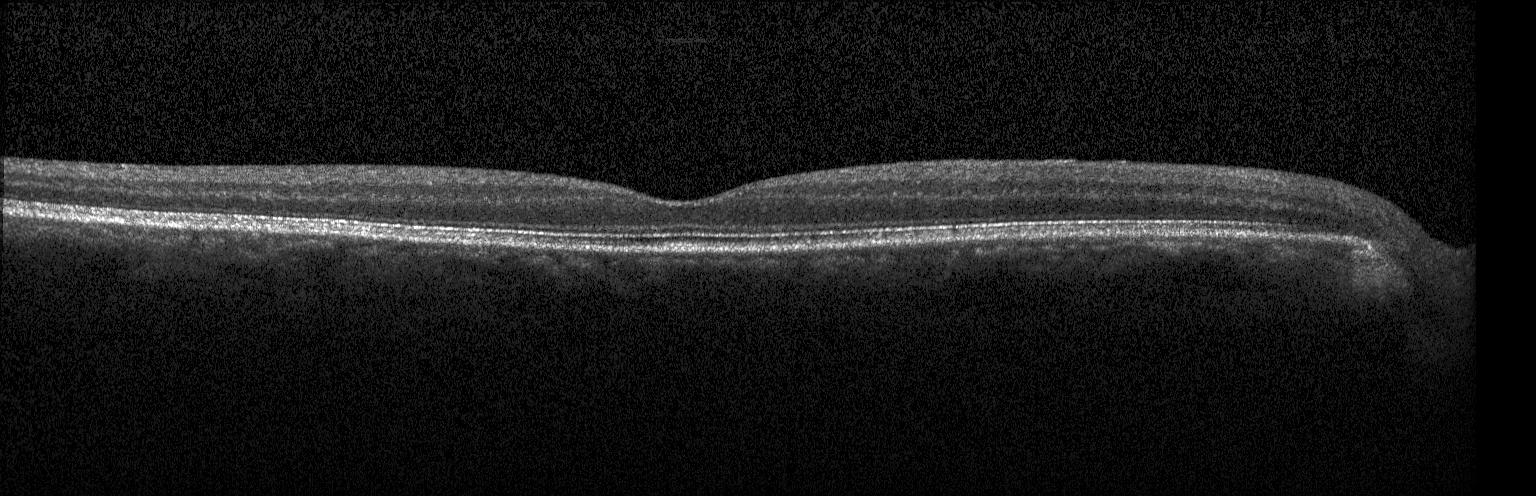
Optical coherence tomography scan · macular scan · instrument: Heidelberg Spectralis.
Impression: neither choroidal neovascularization, diabetic macular edema, nor drusen.